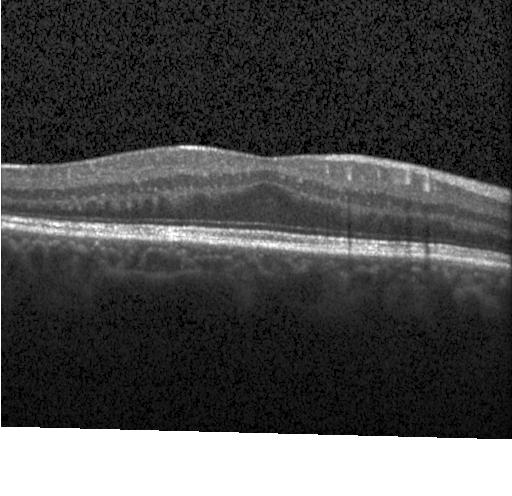 Fovea-centered. Retinal OCT B-scan.
Impression: no evidence of choroidal neovascularization, diabetic macular edema, or drusen.